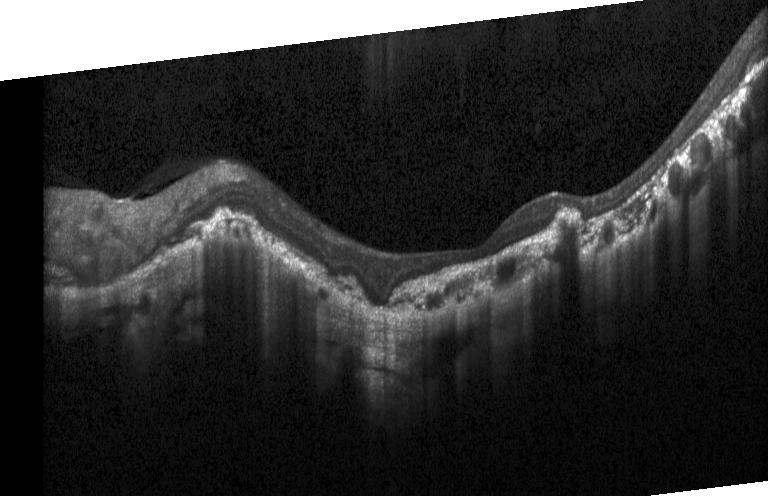 The scan shows CNV.